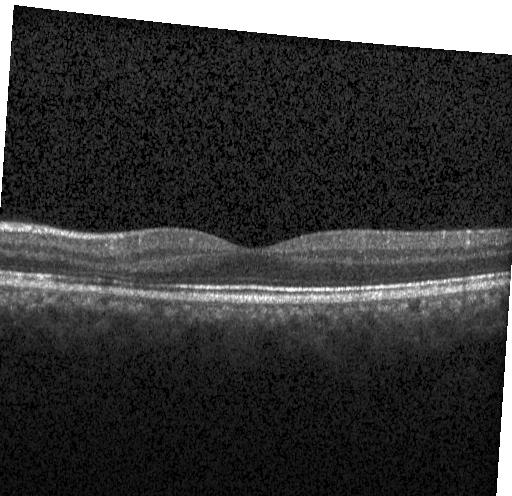 Retinal OCT cross-section · macular scan · acquired on a Heidelberg Spectralis · spectral-domain OCT.
Assessment: neither CNV, DME, nor drusen.